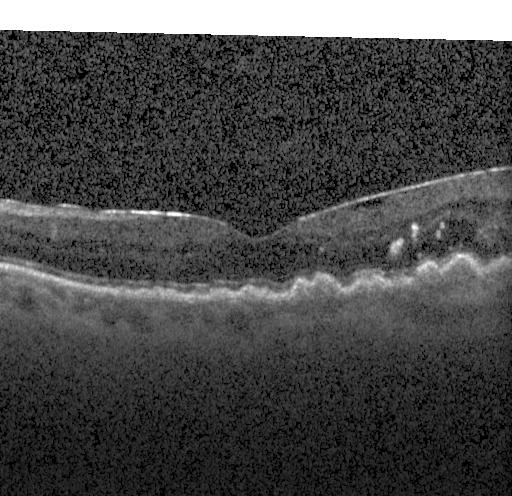 Assessment: sub-RPE drusenoid deposits.